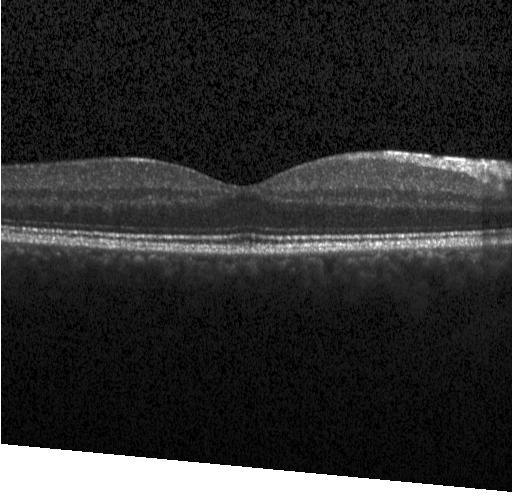
Spectral-domain optical coherence tomography. Instrument: Heidelberg Spectralis. OCT B-scan. The scan shows no evidence of CNV, DME, or drusen.